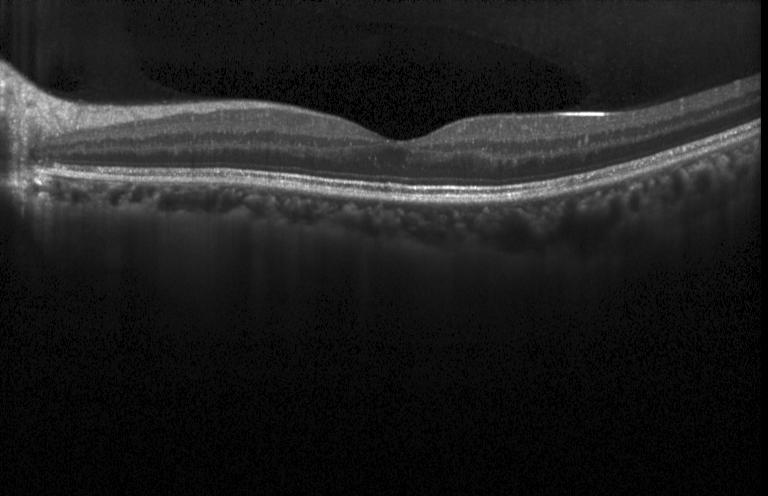
Optical coherence tomography scan. Horizontal scan through the fovea. SD-OCT.
Diagnosis: no evidence of choroidal neovascularization, diabetic macular edema, or drusen.